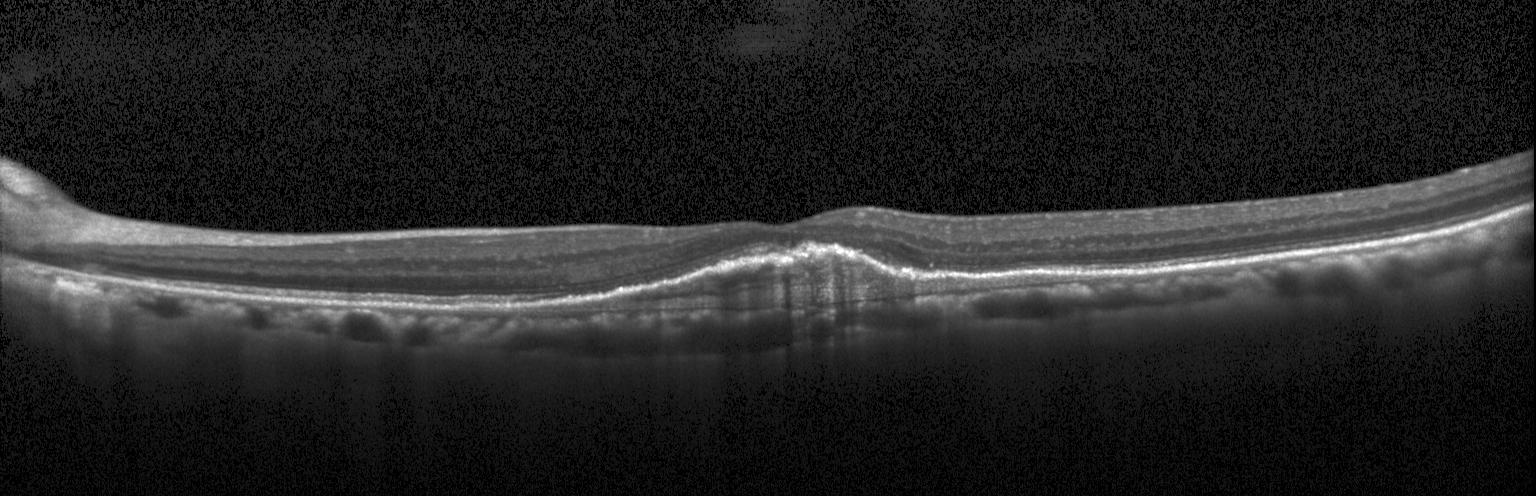 Heidelberg Spectralis OCT system · optical coherence tomography scan · fovea-centered
This B-scan demonstrates choroidal neovascularization (CNV).